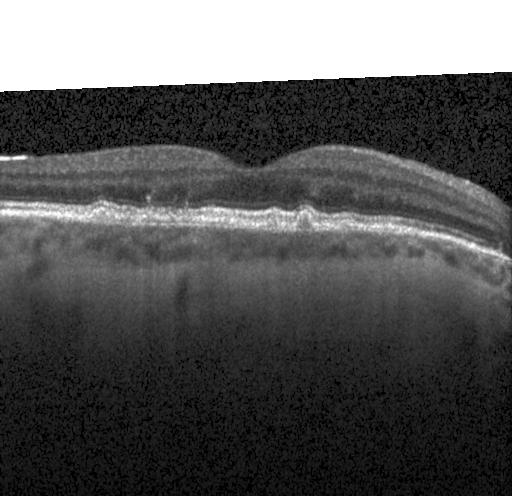 Horizontal scan through the fovea · retinal OCT cross-section. Dx: sub-RPE drusenoid deposits.